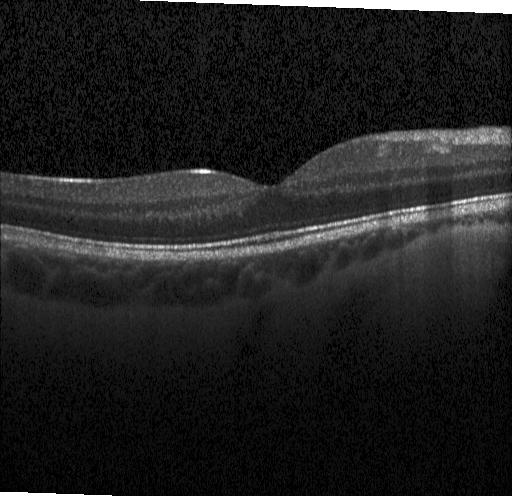
OCT scan showing no CNV, DME, or drusen.